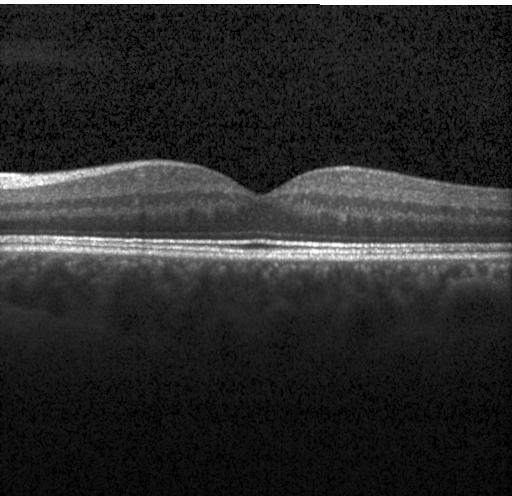

Retinal OCT cross-section. Spectral-domain optical coherence tomography. Centered on the fovea. Heidelberg Spectralis OCT system — Diagnosis: no choroidal neovascularization, no diabetic macular edema, and no drusen.